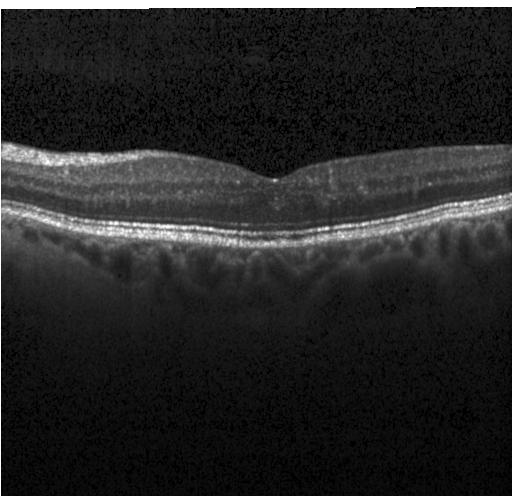 Optical coherence tomography B-scan, Heidelberg Spectralis OCT system, spectral-domain OCT, fovea-centered. Assessment: no choroidal neovascularization, diabetic macular edema, or drusen.